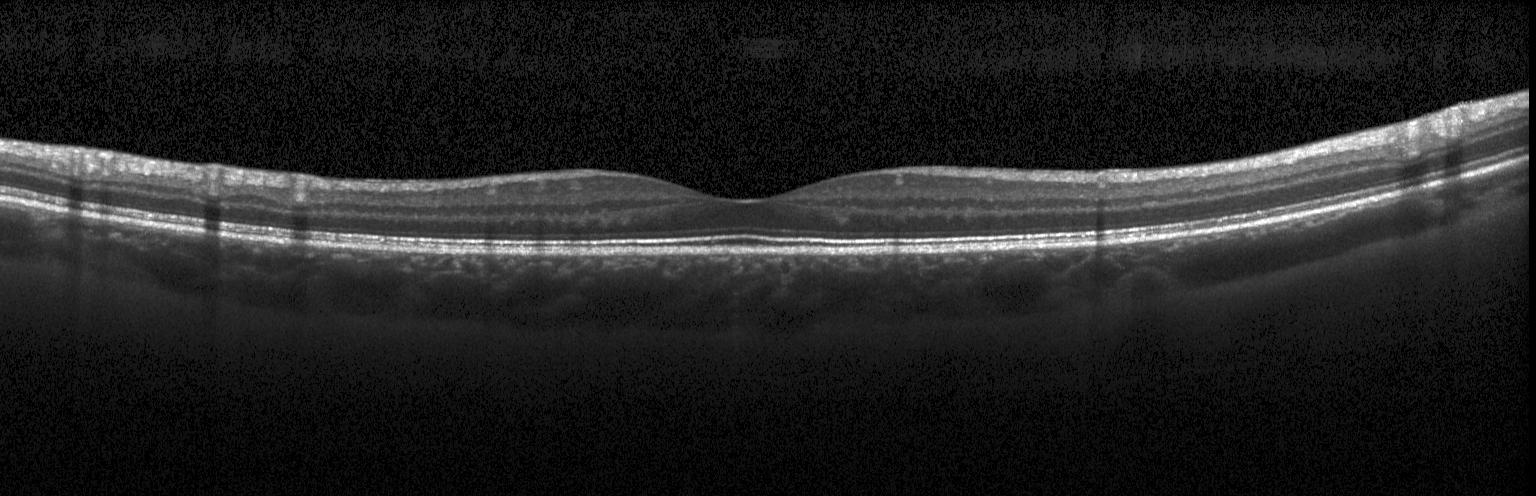
Finding: no CNV, no DME, and no drusen.